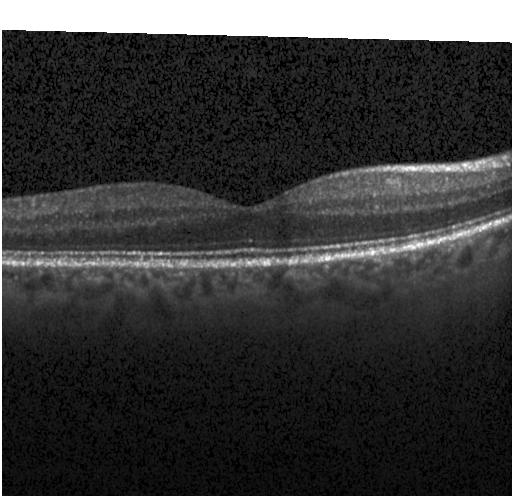

The scan shows no evidence of CNV, DME, or drusen.